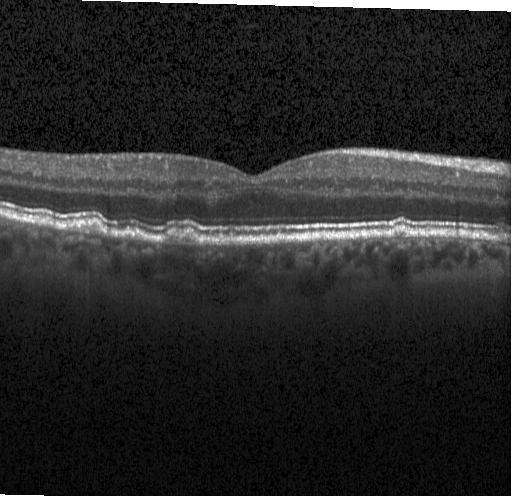
Retinal OCT cross-section showing drusen.